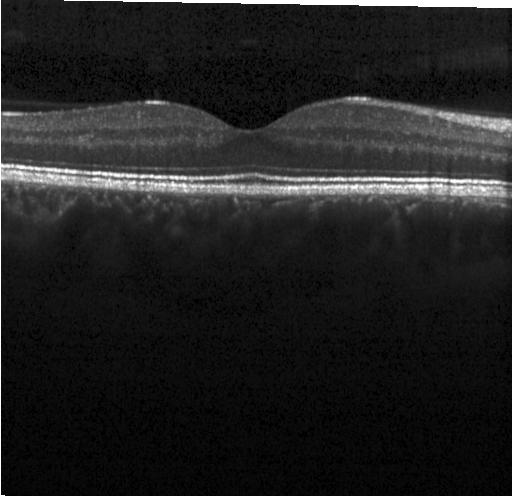 Diagnosis: neither CNV, DME, nor drusen.